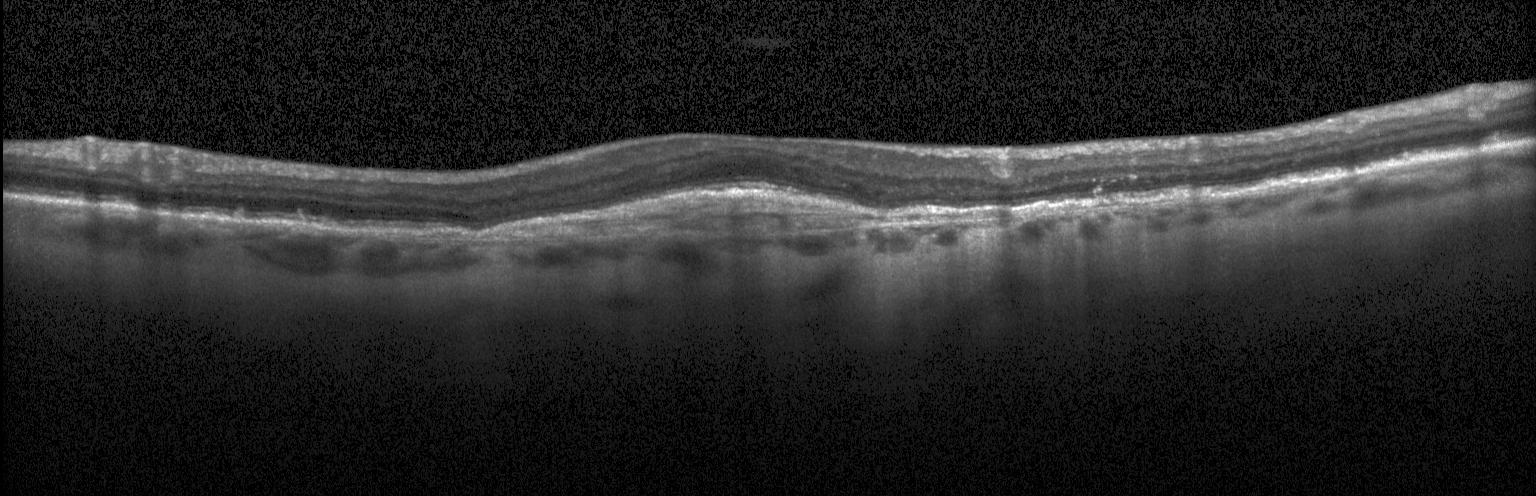

Impression: CNV.